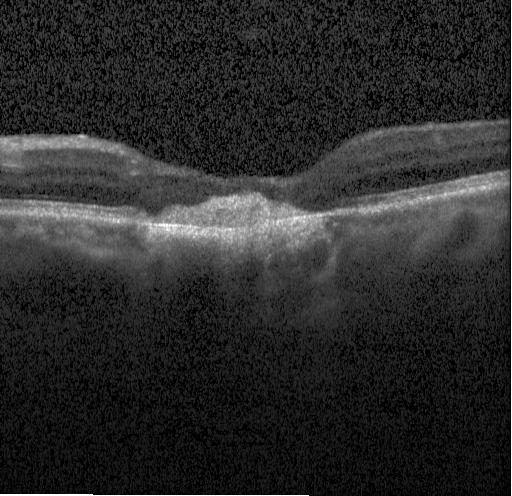 OCT line scan, acquired on a Heidelberg Spectralis, SD-OCT, fovea-centered — Finding: a choroidal neovascular membrane.